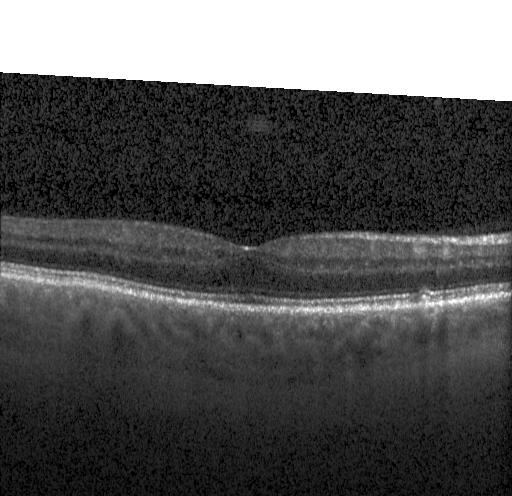
Centered on the fovea. Spectral-domain optical coherence tomography. Heidelberg Spectralis. Retinal OCT cross-section.
Finding: no choroidal neovascularization, no diabetic macular edema, and no drusen.